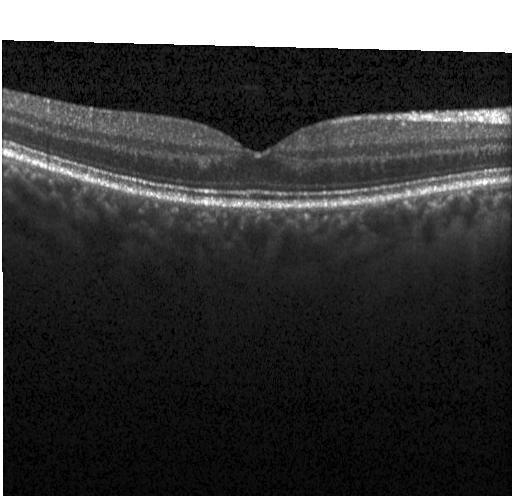

Macular OCT demonstrating neither choroidal neovascularization, diabetic macular edema, nor drusen.